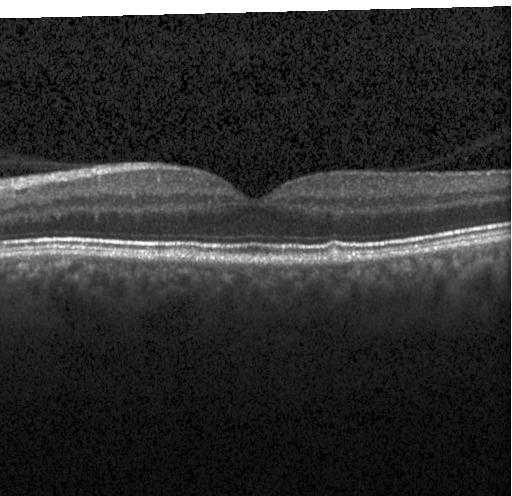 OCT finding: multiple drusen.